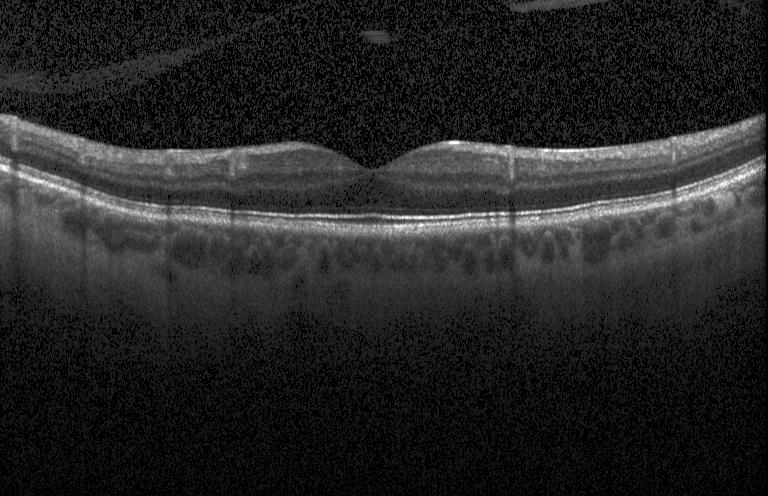
Acquired on a Heidelberg Spectralis, retinal OCT cross-section, spectral-domain optical coherence tomography. Dx: no CNV, DME, or drusen.